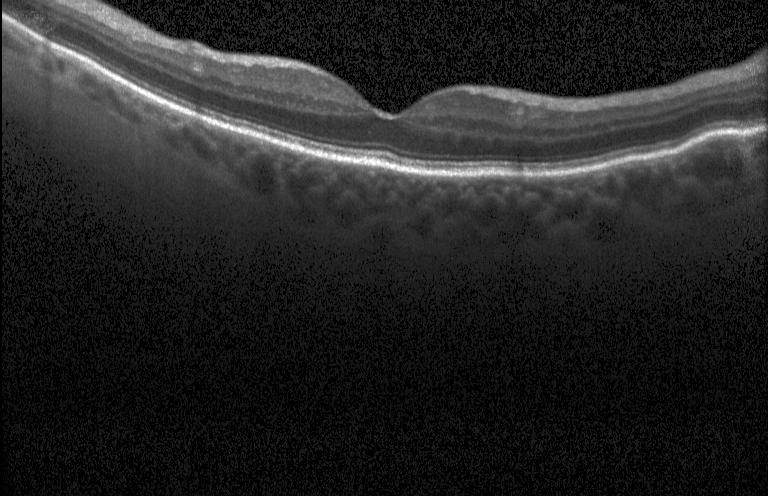 Diagnosis: no evidence of choroidal neovascularization, diabetic macular edema, or drusen.